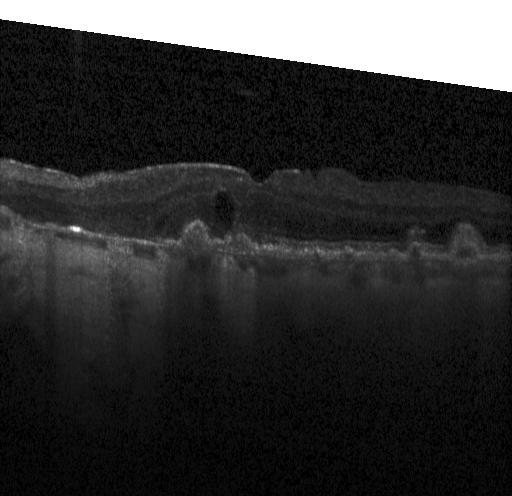
Optical coherence tomography B-scan · centered on the fovea · Heidelberg Spectralis · spectral-domain OCT. Impression: choroidal neovascularization.